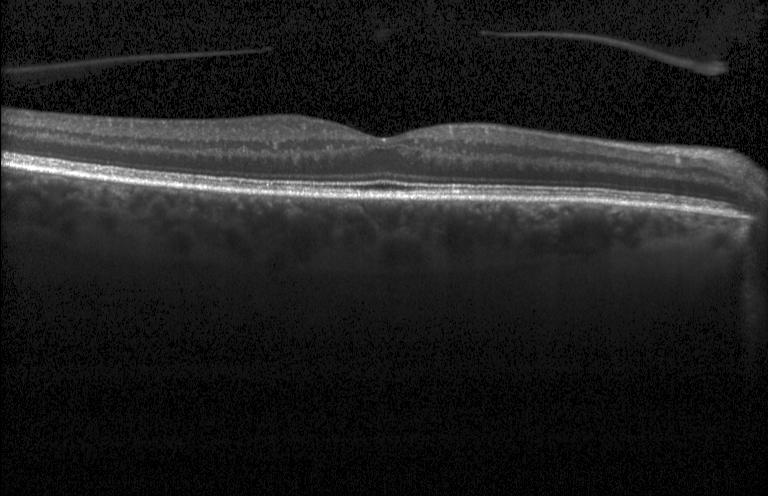
OCT line scan · centered on the fovea
Impression: no choroidal neovascularization, no diabetic macular edema, and no drusen.